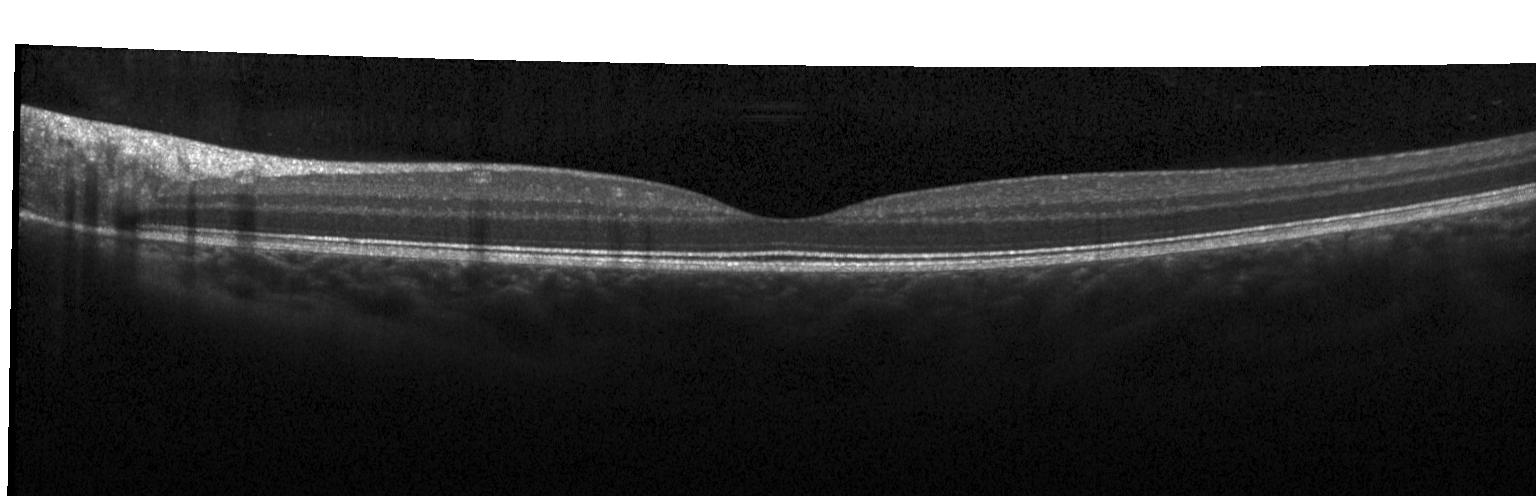
Impression: neither choroidal neovascularization, diabetic macular edema, nor drusen.